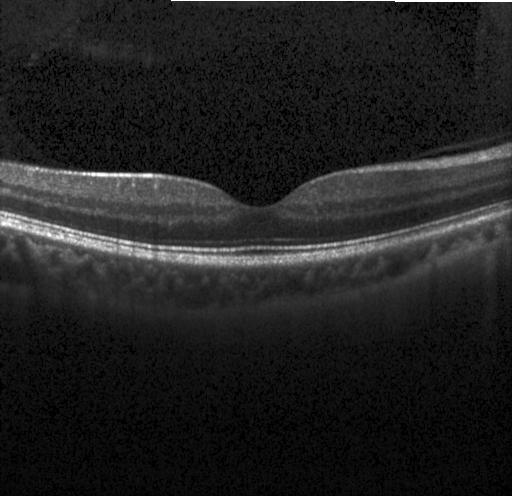
Retinal OCT cross-section · macular scan
Diagnosis: no choroidal neovascularization, diabetic macular edema, or drusen.